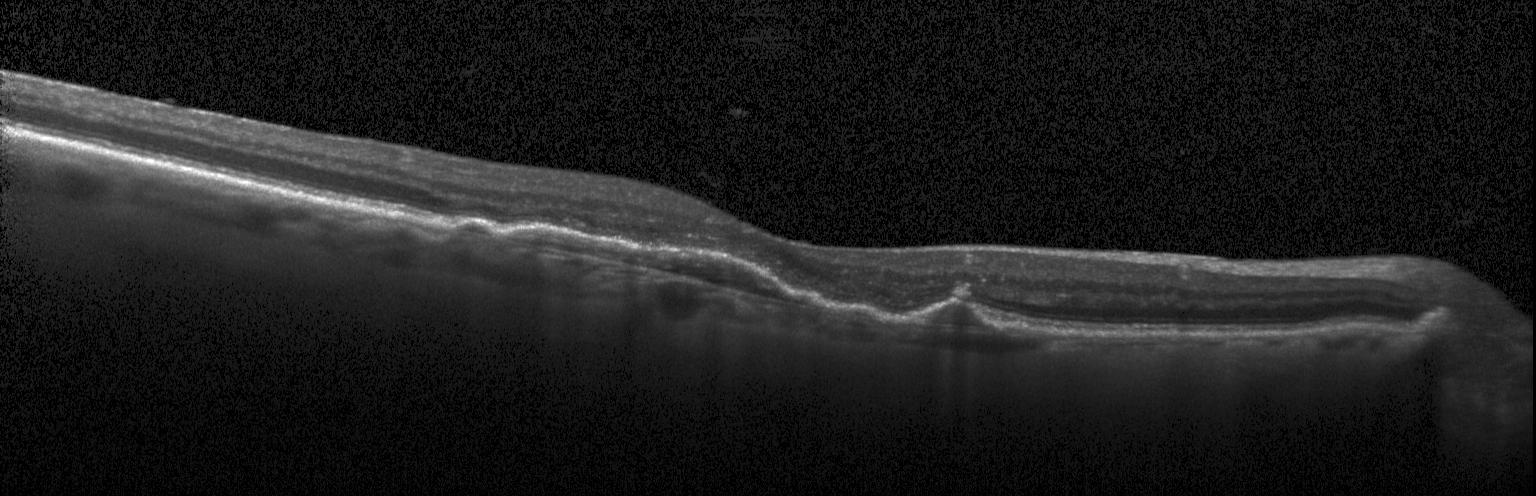 OCT line scan. Macular OCT: a choroidal neovascular membrane.